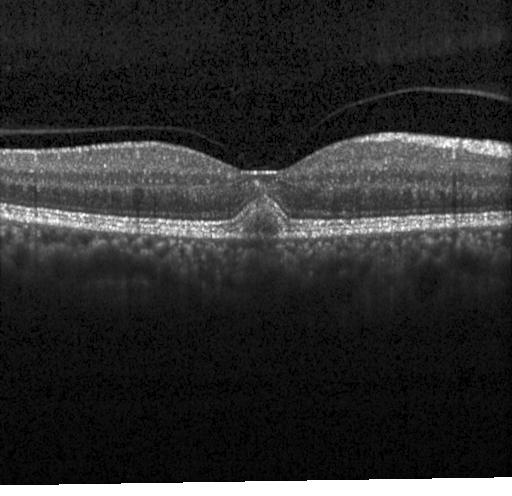

OCT scan showing a choroidal neovascular membrane.